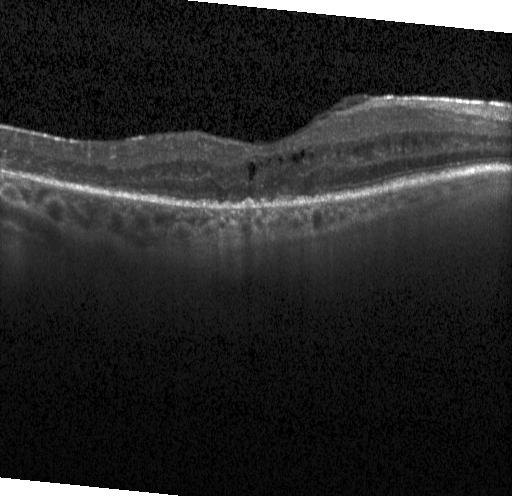
Centered on the fovea, optical coherence tomography B-scan — Assessment: DME.